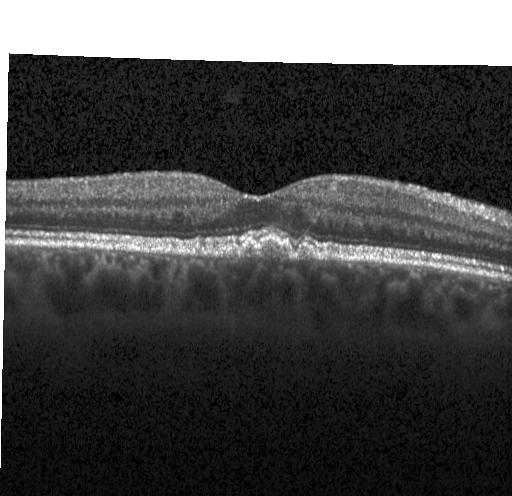
Optical coherence tomography scan, through the macula, Heidelberg Spectralis OCT system — Finding: drusen.